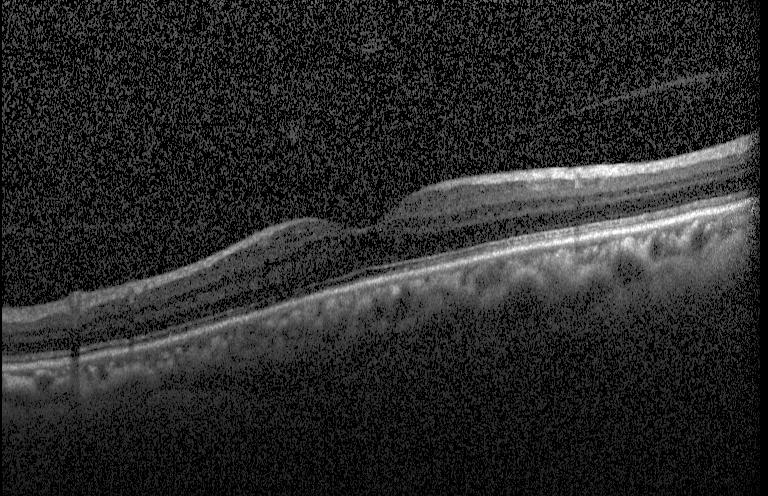
Optical coherence tomography B-scan. Assessment: no CNV, no DME, and no drusen.